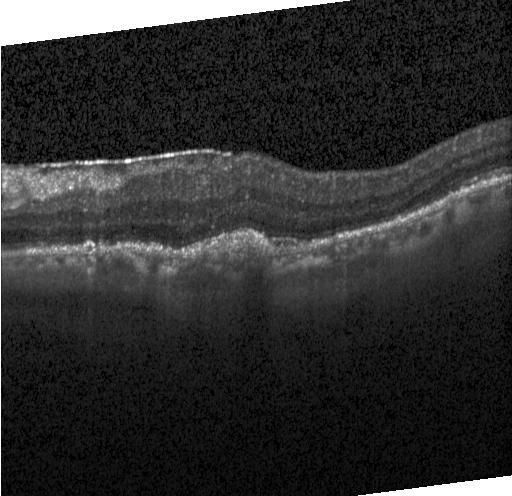

Heidelberg Spectralis OCT system; OCT line scan
The scan shows choroidal neovascularization (CNV).